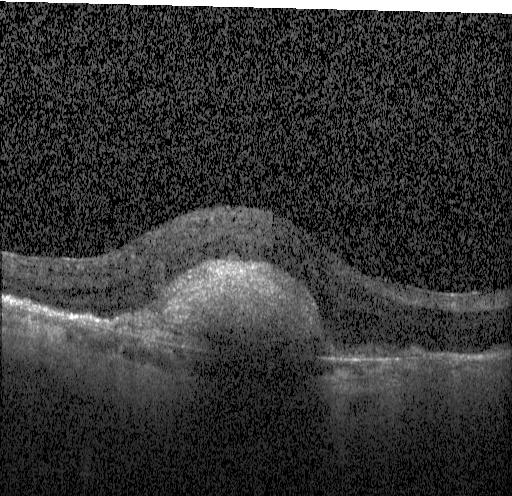
Spectral-domain OCT B-scan: a choroidal neovascular membrane.